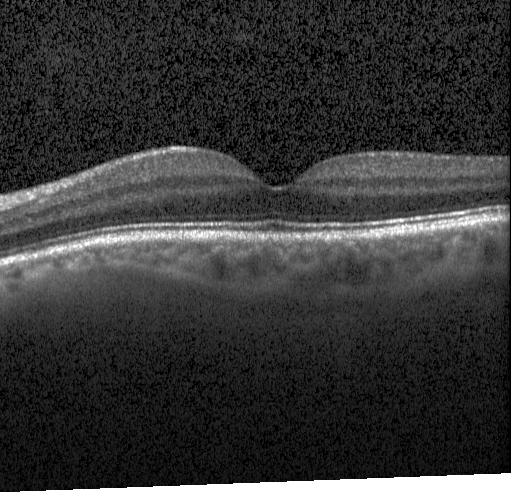

Impression: no CNV, DME, or drusen.